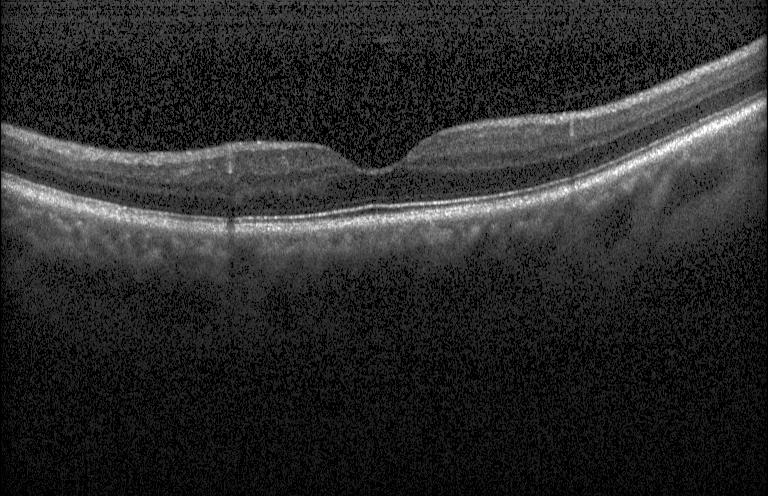

Spectral-domain optical coherence tomography; OCT line scan; fovea-centered.
Impression: no choroidal neovascularization, no diabetic macular edema, and no drusen.